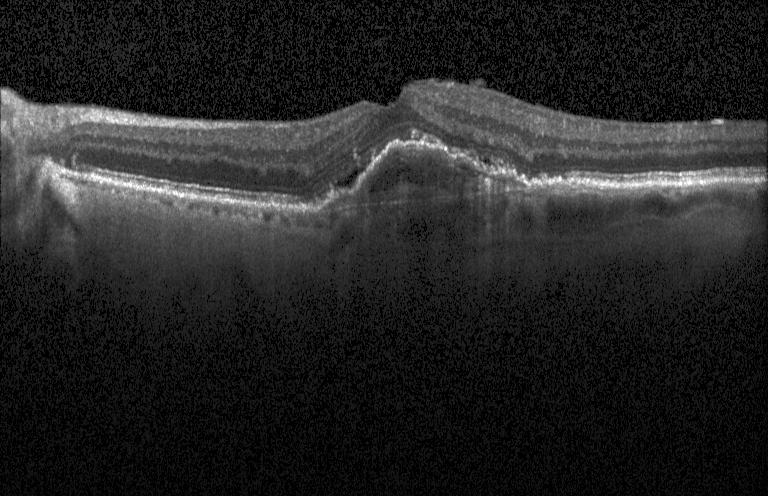
Spectral-domain OCT; instrument: Heidelberg Spectralis; through the macula; retinal OCT B-scan — This B-scan demonstrates a choroidal neovascular membrane.